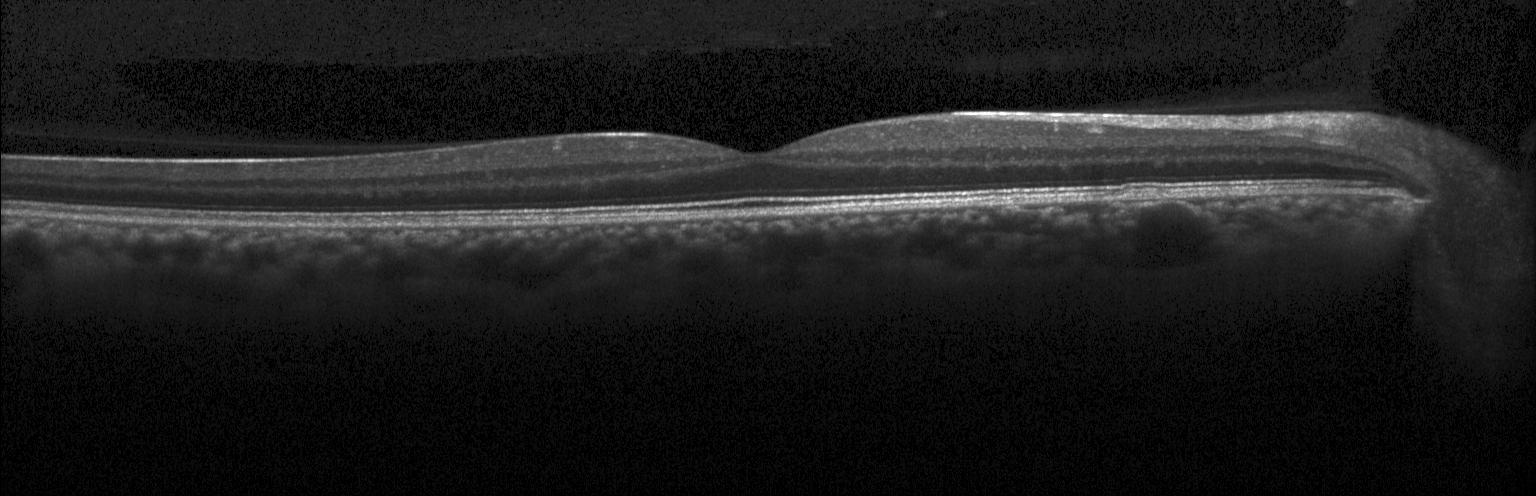 Retinal OCT cross-section.
This B-scan demonstrates neither CNV, DME, nor drusen.